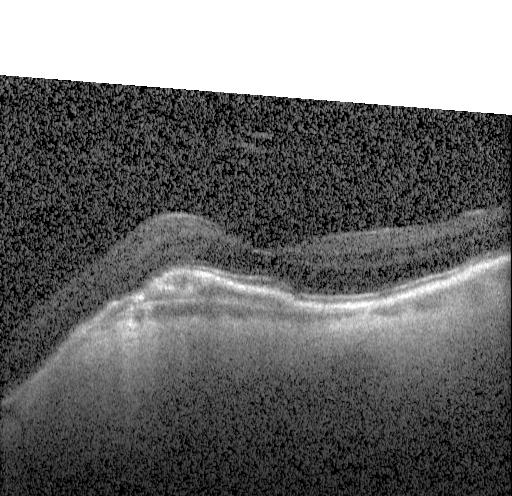

Diagnosis: a choroidal neovascular membrane.